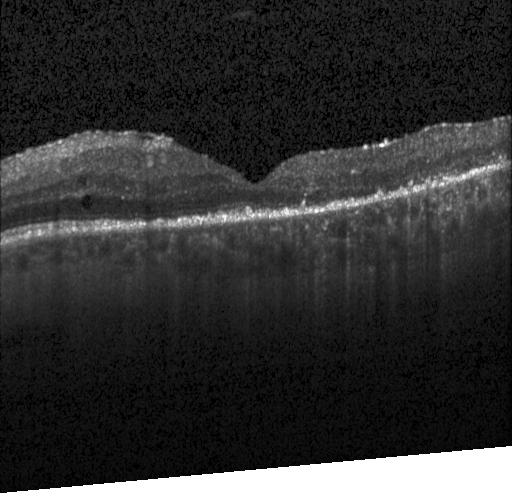

Diagnosis: DME.